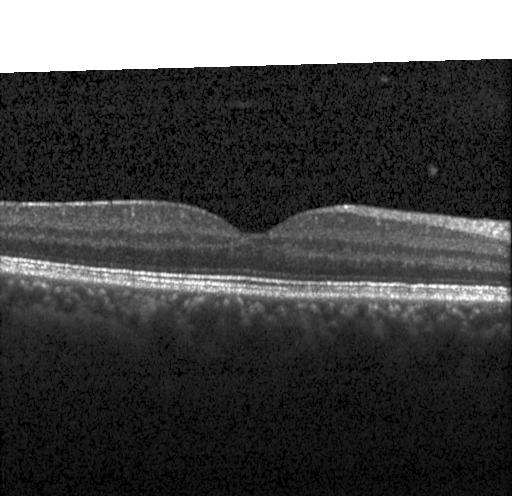

This B-scan demonstrates no evidence of choroidal neovascularization, diabetic macular edema, or drusen.